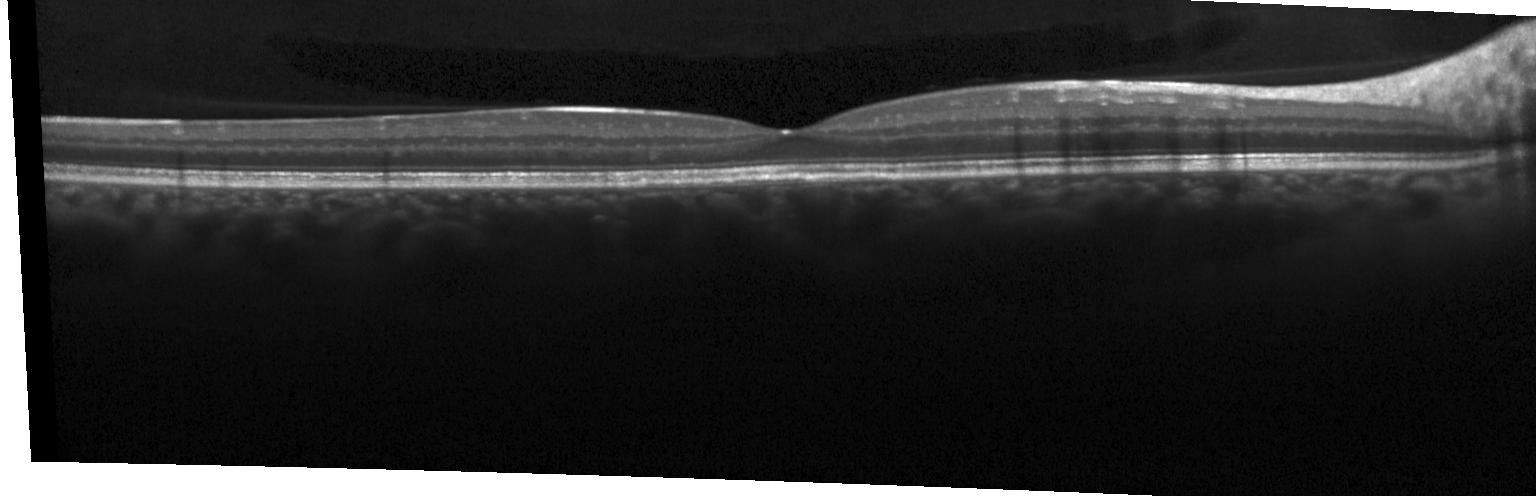
OCT B-scan.
OCT finding: no choroidal neovascularization, no diabetic macular edema, and no drusen.